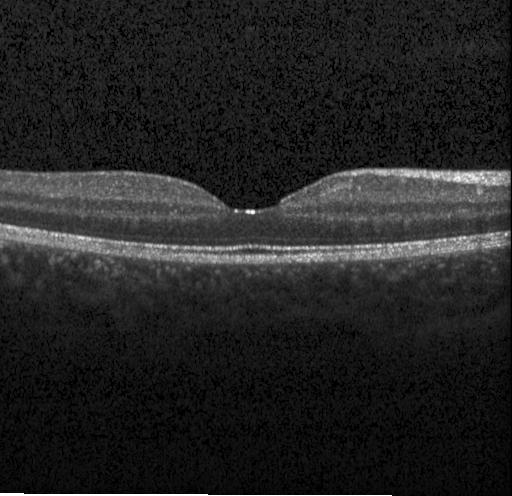

Impression: no evidence of choroidal neovascularization, diabetic macular edema, or drusen.